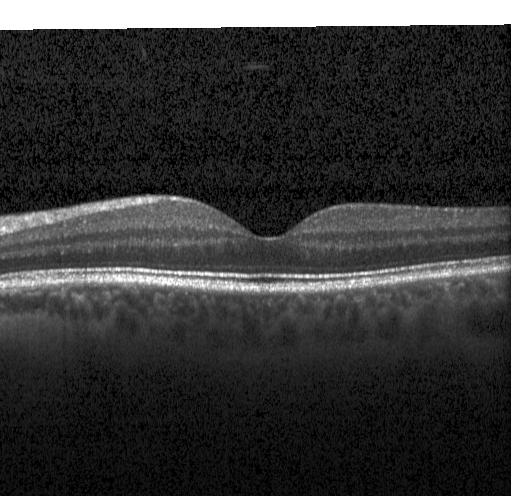 Finding: no CNV, DME, or drusen.